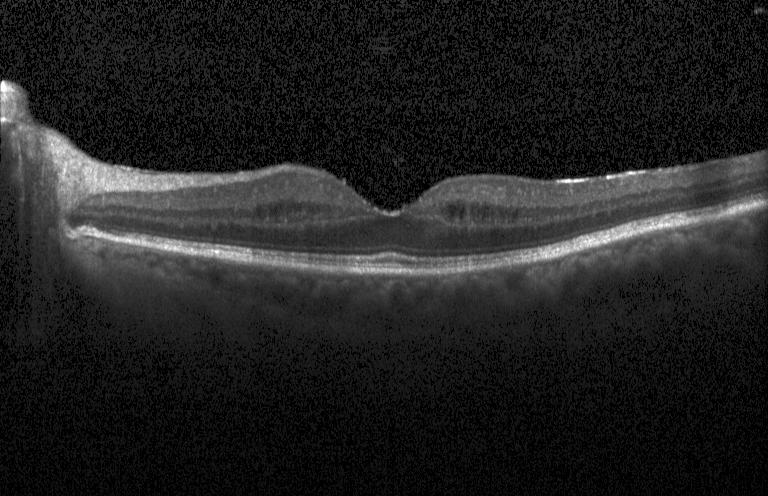
Retinal OCT cross-section; Heidelberg Spectralis.
Finding: diabetic macular edema (DME).